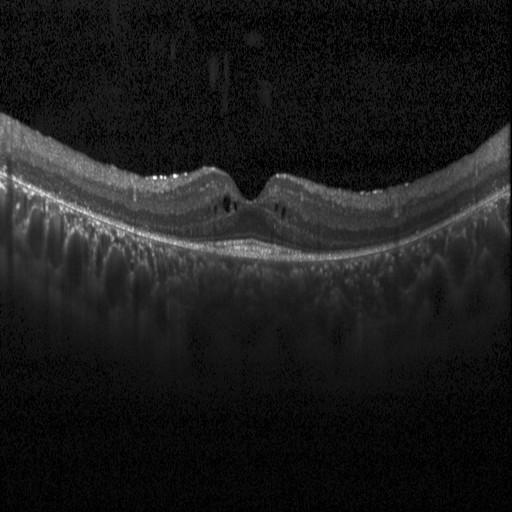

Macular OCT demonstrating diabetic macular edema.